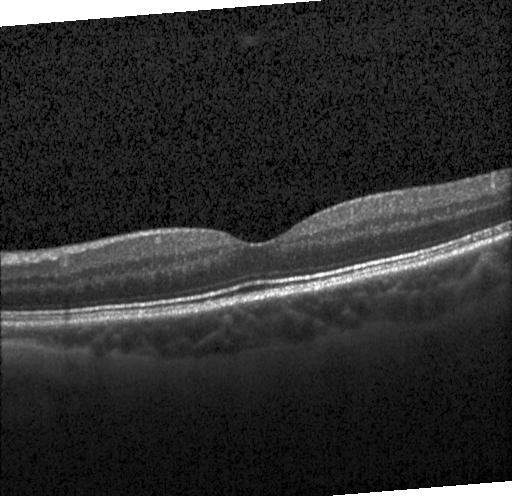 OCT B-scan · SD-OCT.
Diagnosis: no evidence of CNV, DME, or drusen.